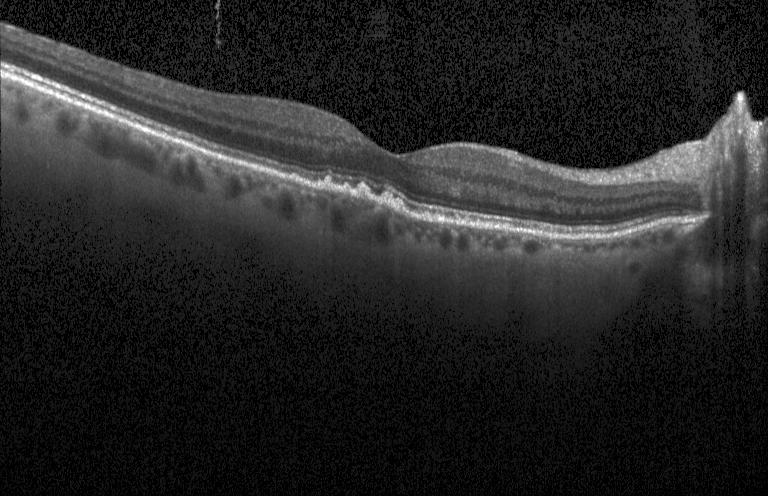 Finding: drusen.